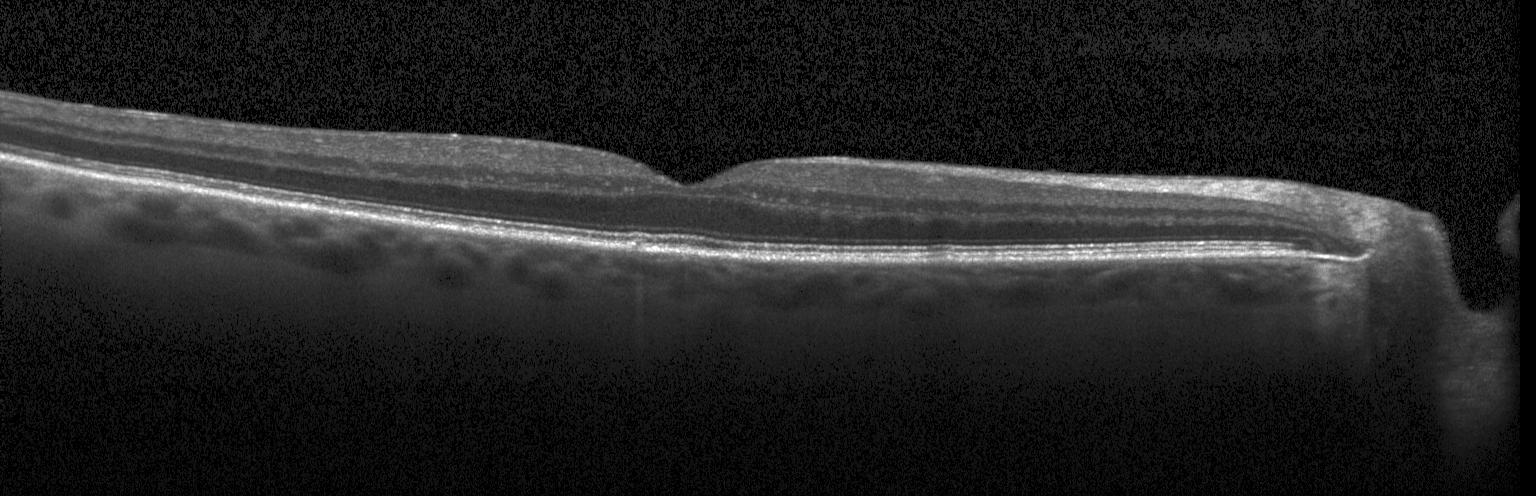
Horizontal scan through the fovea, Heidelberg Spectralis, optical coherence tomography scan — This B-scan demonstrates no CNV, no DME, and no drusen.